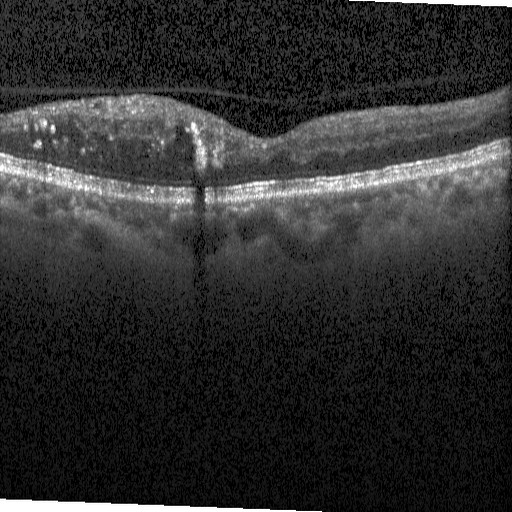

Optical coherence tomography B-scan, fovea-centered. Finding: diabetic macular edema.